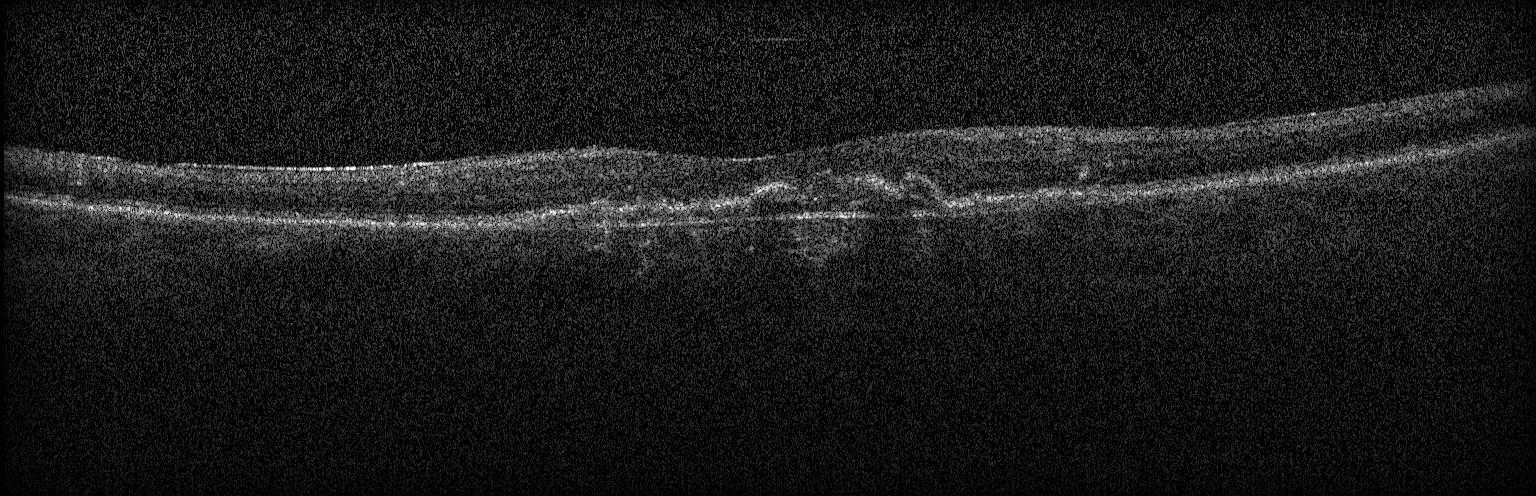

Acquired on a Heidelberg Spectralis, retinal OCT cross-section. Impression: a choroidal neovascular membrane.